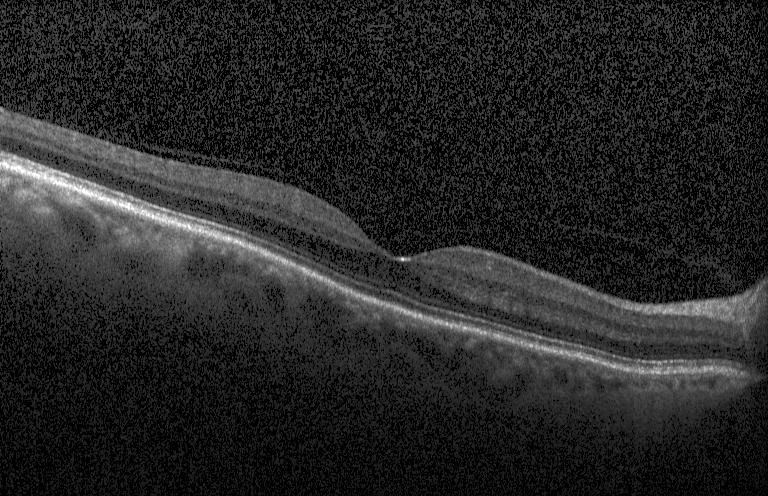 OCT line scan.
OCT finding: neither choroidal neovascularization, diabetic macular edema, nor drusen.